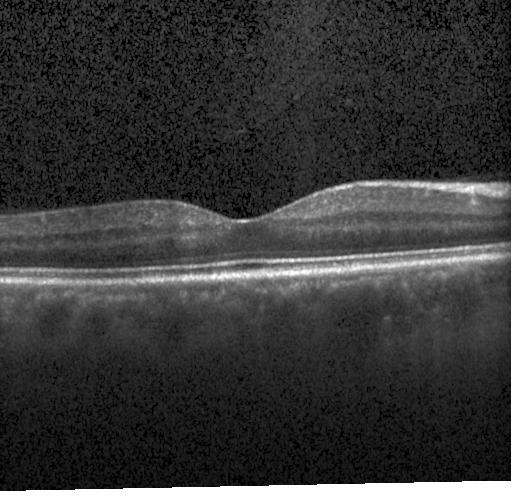 OCT line scan. Centered on the fovea. Spectral-domain OCT. Diagnosis: neither choroidal neovascularization, diabetic macular edema, nor drusen.